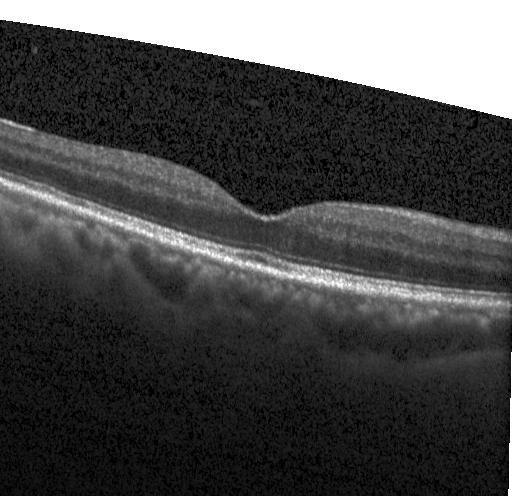
Acquired on a Heidelberg Spectralis; centered on the fovea; SD-OCT; retinal OCT B-scan — The scan shows no choroidal neovascularization, no diabetic macular edema, and no drusen.